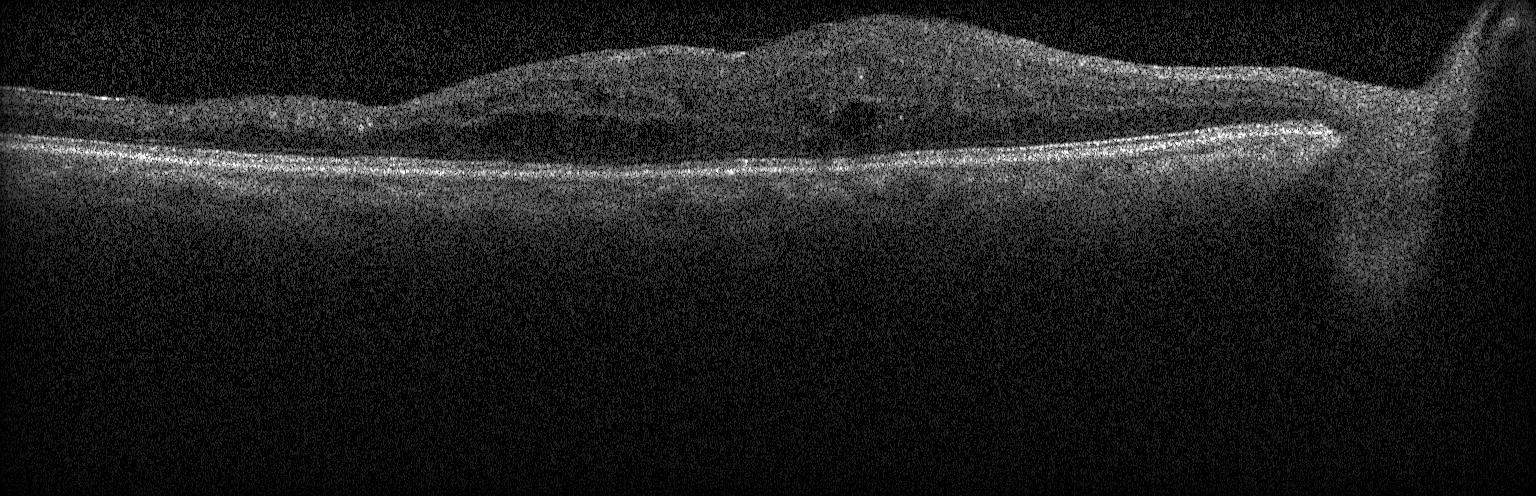 OCT B-scan; Heidelberg Spectralis; macular scan; SD-OCT. Impression: DME.